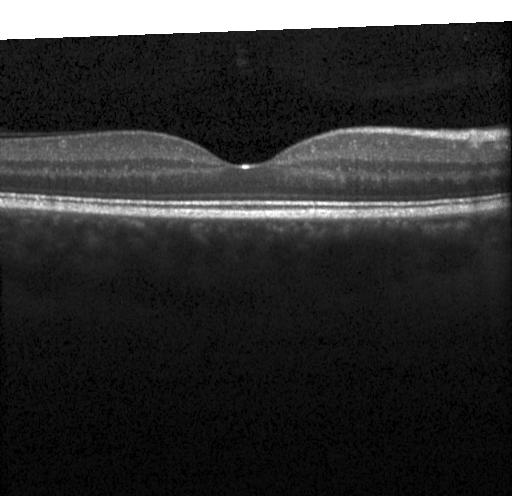 Impression: no evidence of choroidal neovascularization, diabetic macular edema, or drusen.